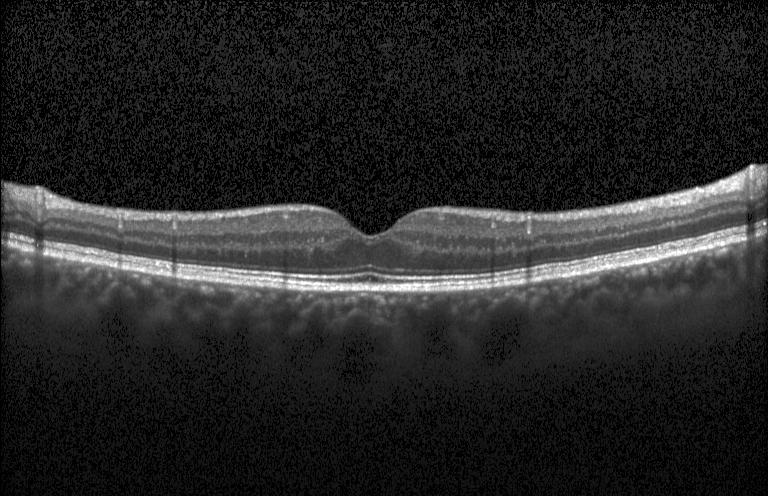
Spectral-domain OCT, Heidelberg Spectralis OCT system, through the macula, optical coherence tomography B-scan
The scan shows no choroidal neovascularization, no diabetic macular edema, and no drusen.